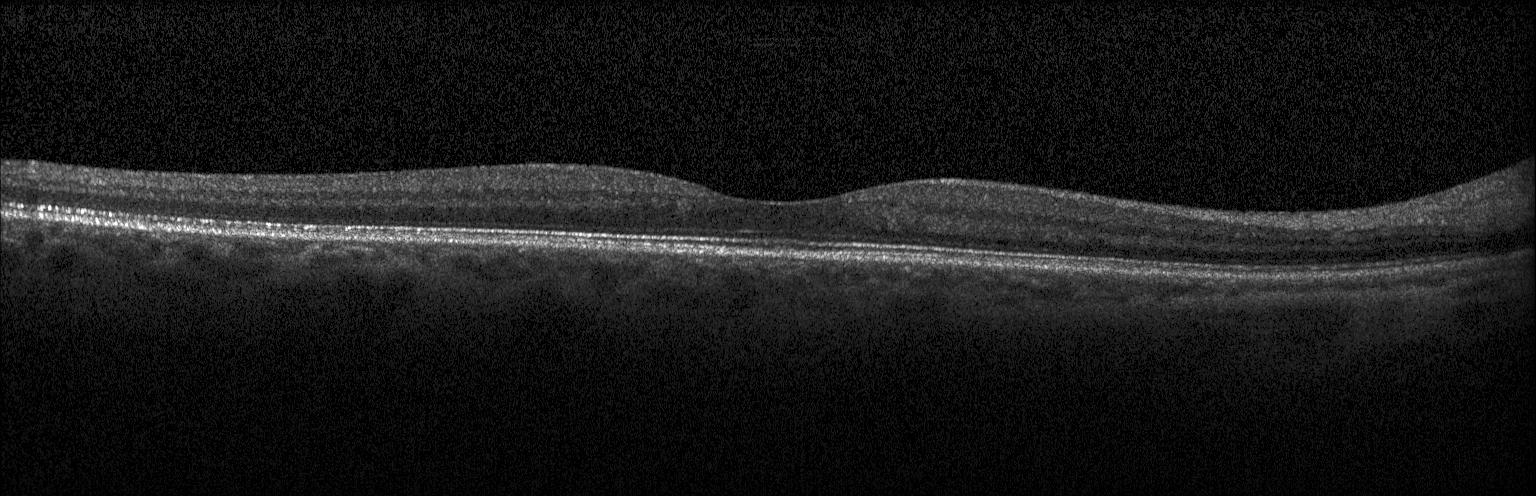 Diagnosis: no evidence of choroidal neovascularization, diabetic macular edema, or drusen.